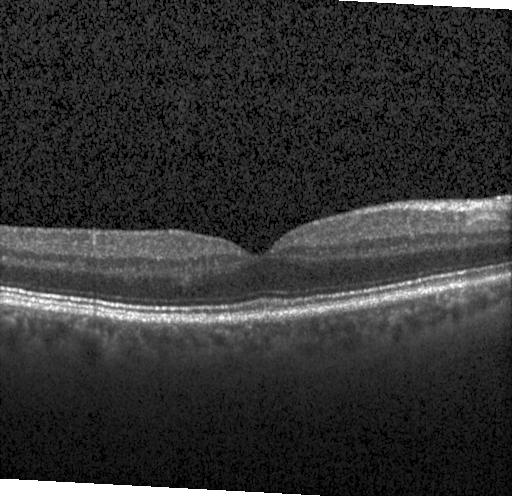

Horizontal scan through the fovea · retinal OCT cross-section · acquired on a Heidelberg Spectralis — Finding: no CNV, no DME, and no drusen.